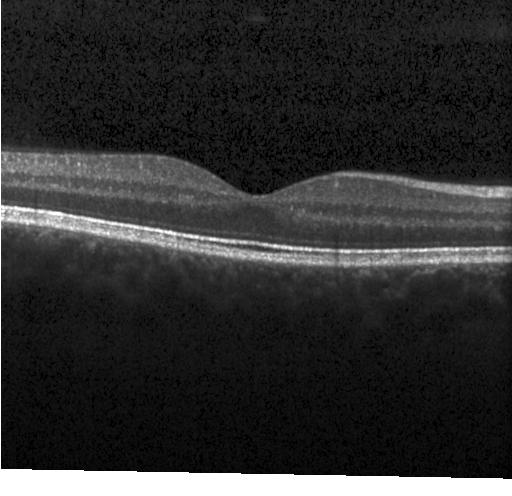

Optical coherence tomography B-scan. Macular scan — Macular OCT: no choroidal neovascularization, no diabetic macular edema, and no drusen.